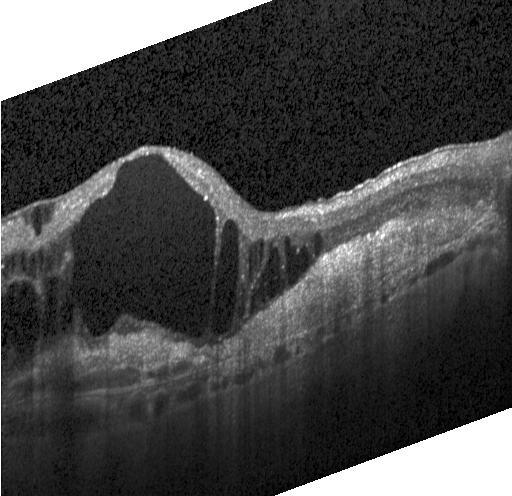

Retinal OCT B-scan; spectral-domain optical coherence tomography; acquired on a Heidelberg Spectralis.
Diagnosis: choroidal neovascularization (CNV).